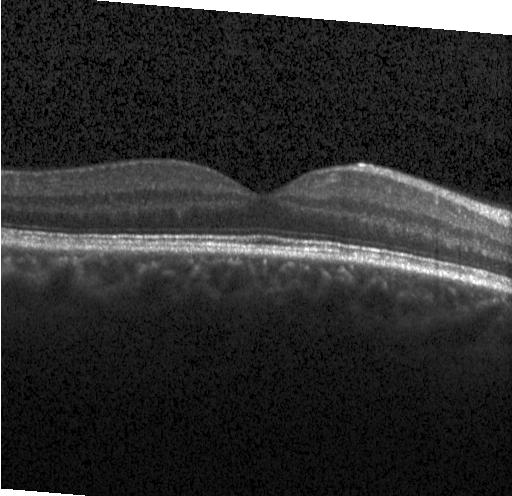
Acquired on a Heidelberg Spectralis, macular scan, optical coherence tomography scan, spectral-domain OCT.
Diagnosis: neither CNV, DME, nor drusen.